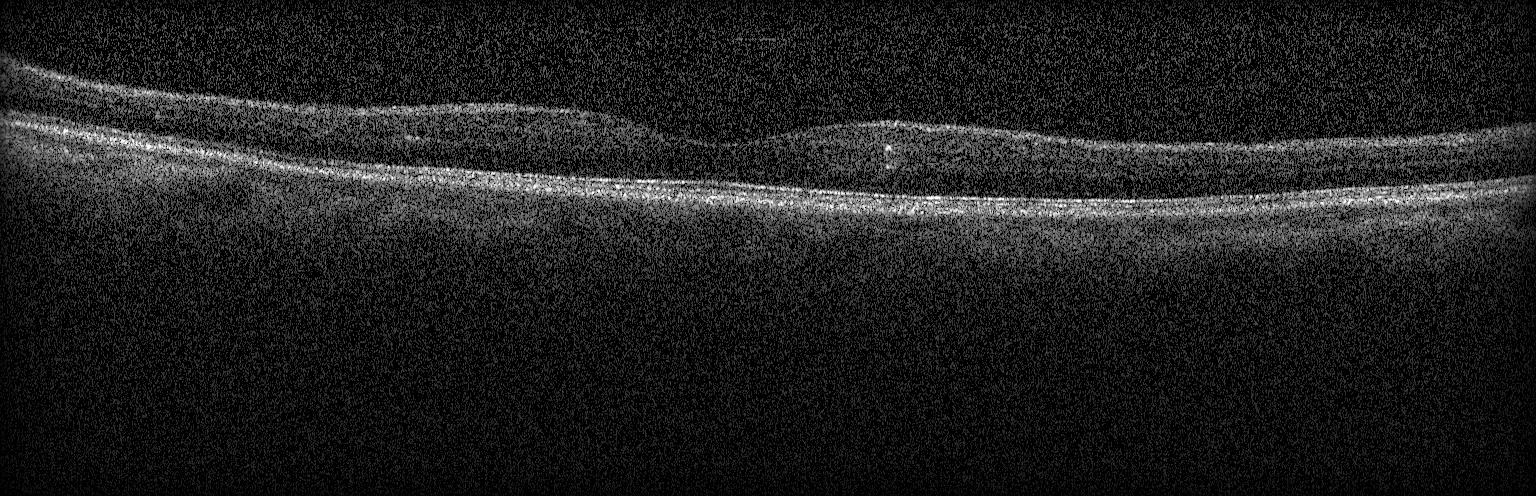

OCT B-scan showing no evidence of choroidal neovascularization, diabetic macular edema, or drusen.